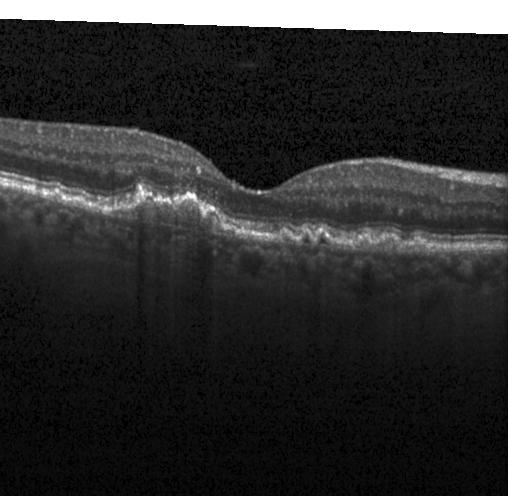
Impression: a choroidal neovascular membrane.